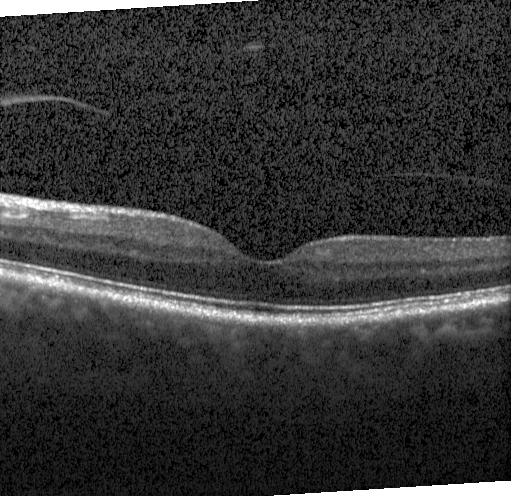
Retinal OCT cross-section
Dx: no choroidal neovascularization, diabetic macular edema, or drusen.